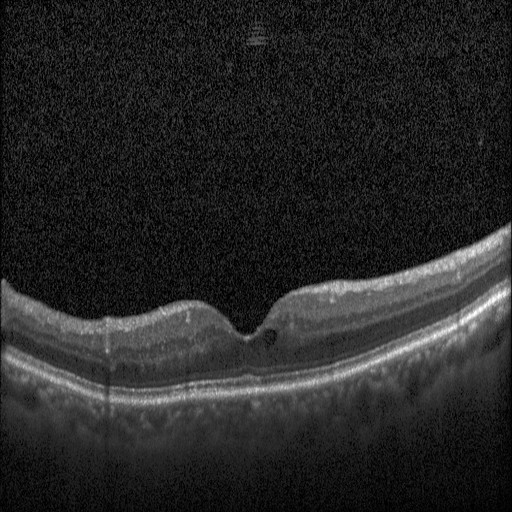

Retinal OCT cross-section
Diagnosis: DME.